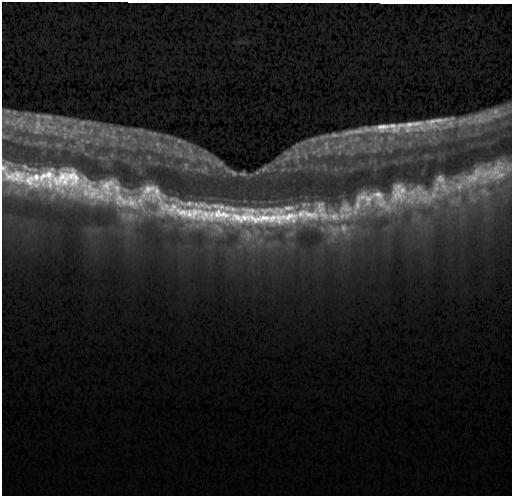

This B-scan demonstrates multiple drusen.